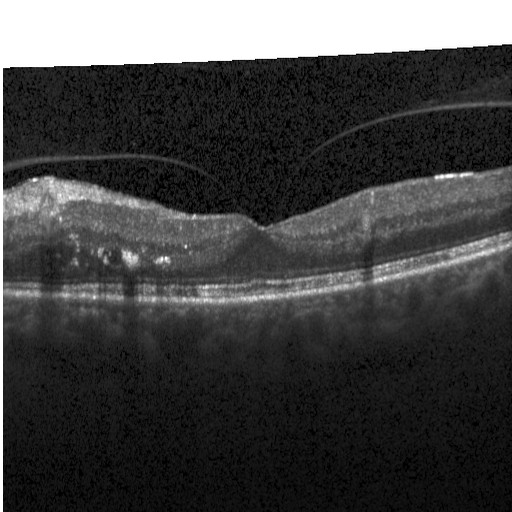
Optical coherence tomography scan.
The scan shows diabetic macular edema.